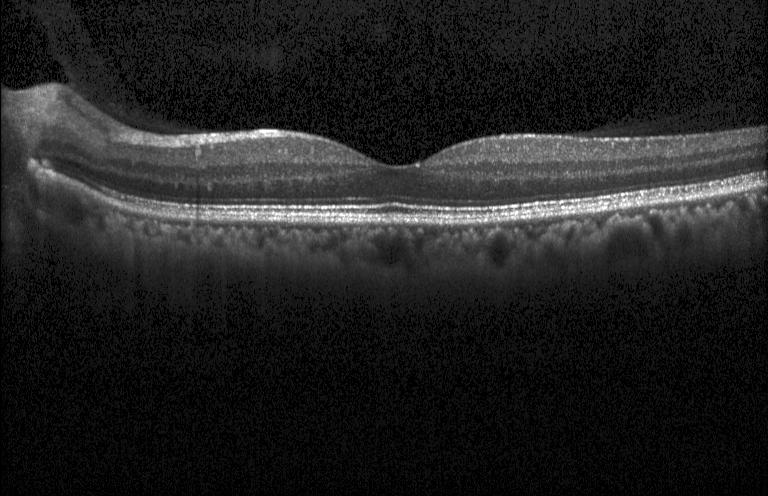

Assessment: no CNV, DME, or drusen.